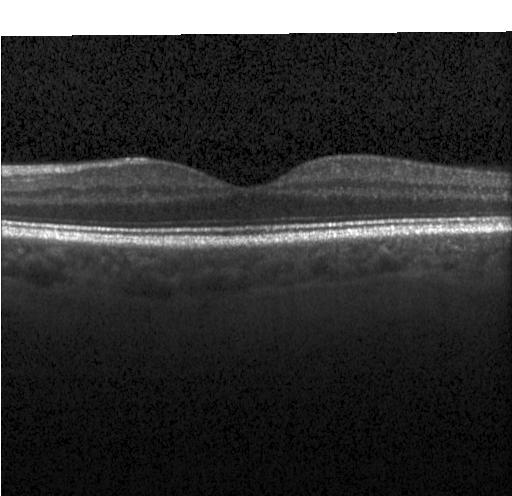 Neither choroidal neovascularization, diabetic macular edema, nor drusen.